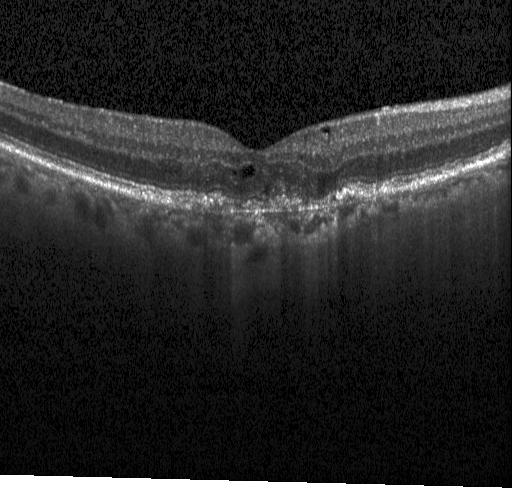

Retinal OCT cross-section. OCT finding: choroidal neovascularization.